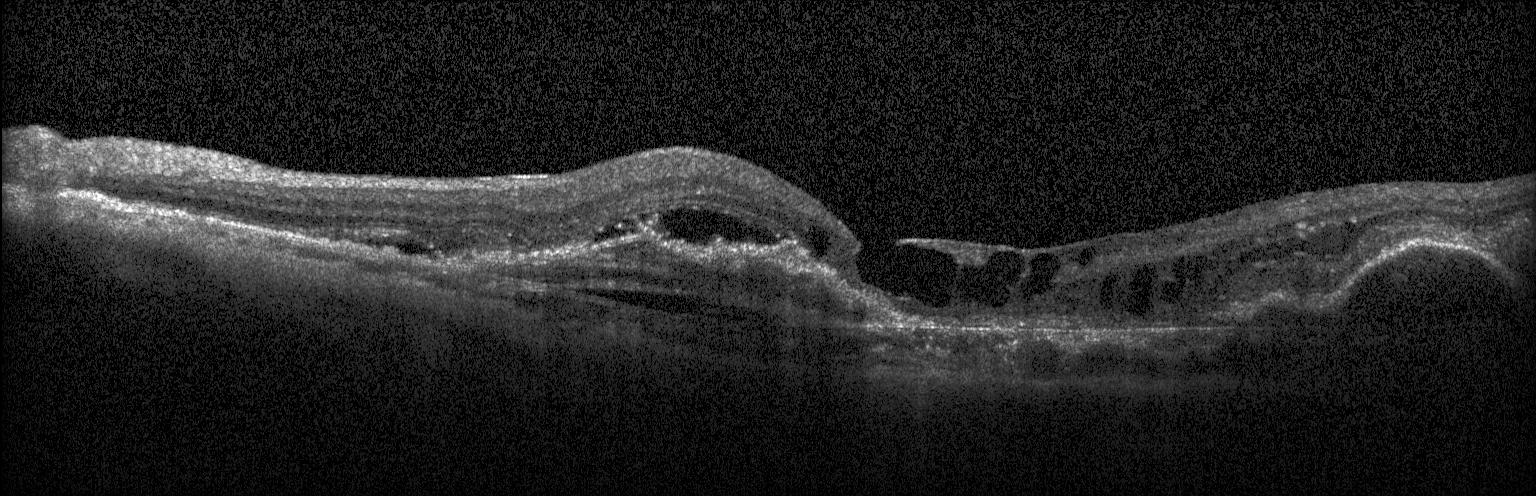
Optical coherence tomography B-scan, instrument: Heidelberg Spectralis, spectral-domain optical coherence tomography
Dx: a choroidal neovascular membrane.